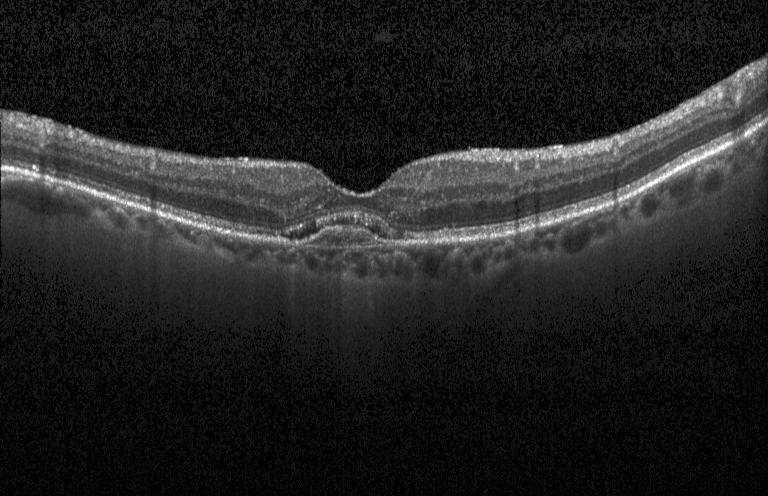
Retinal OCT cross-section showing a choroidal neovascular membrane.